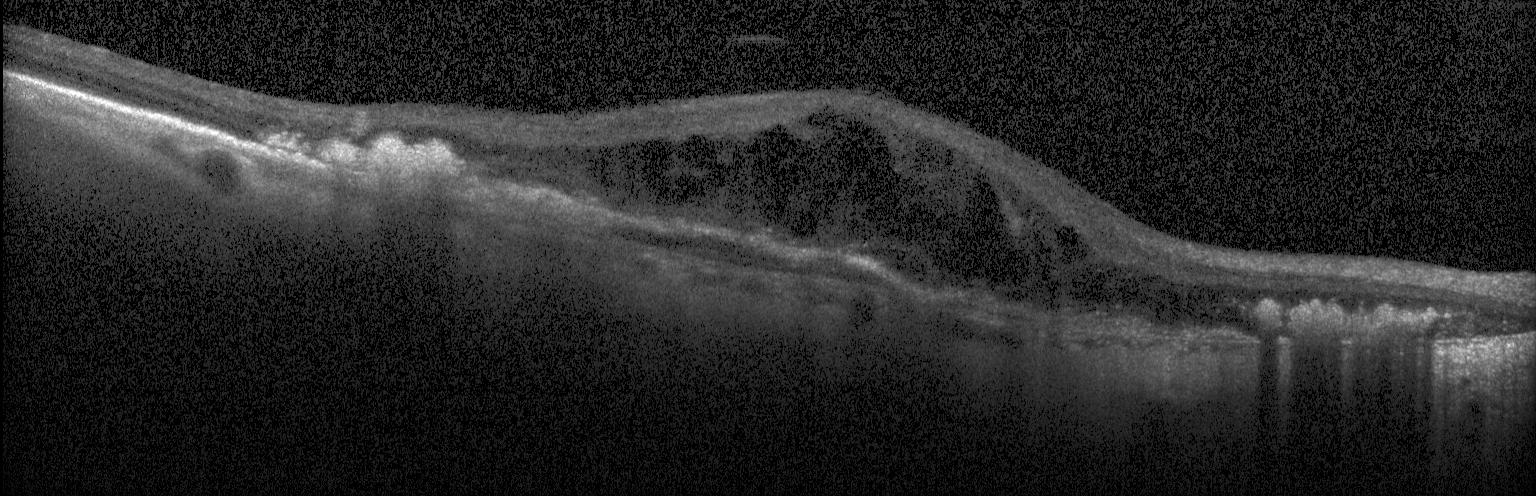 Horizontal scan through the fovea. Spectral-domain optical coherence tomography. Heidelberg Spectralis. Optical coherence tomography scan — This B-scan demonstrates a choroidal neovascular membrane.